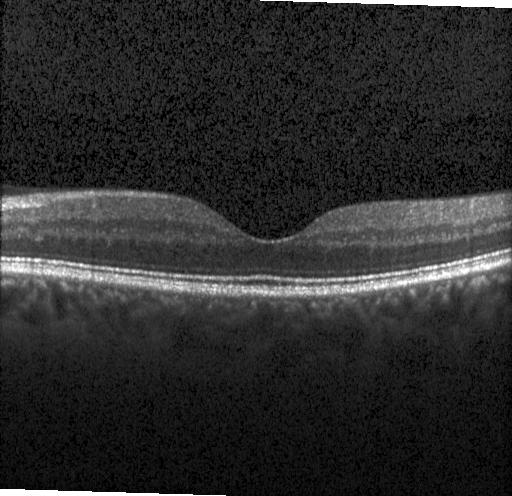

Optical coherence tomography scan — Macular OCT: no CNV, no DME, and no drusen.